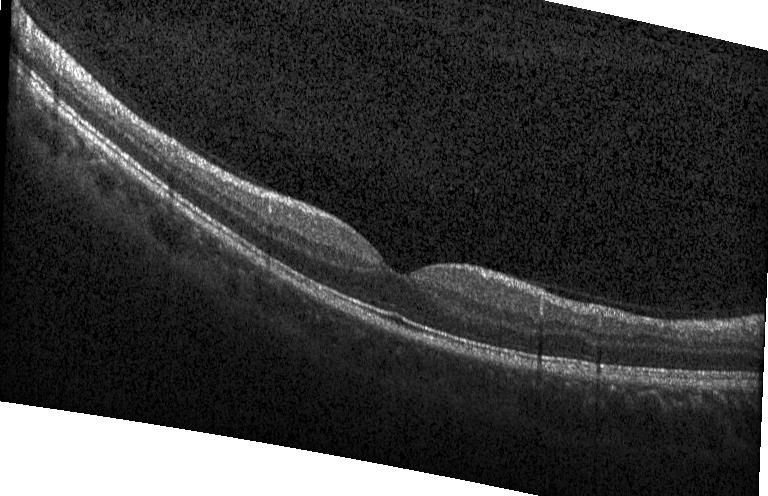 Horizontal scan through the fovea. Heidelberg Spectralis. Retinal OCT cross-section.
Diagnosis: no choroidal neovascularization, no diabetic macular edema, and no drusen.